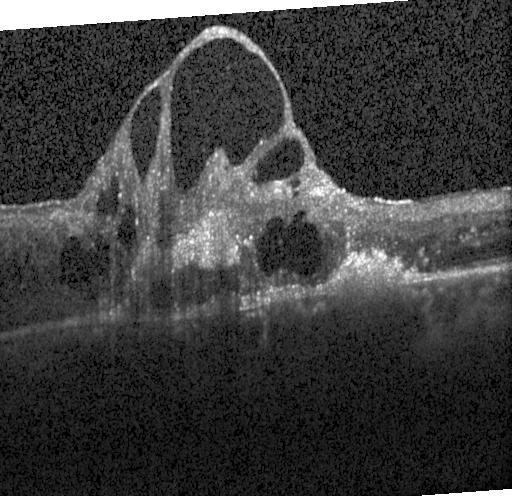 Spectral-domain optical coherence tomography; retinal OCT cross-section
Finding: a choroidal neovascular membrane.